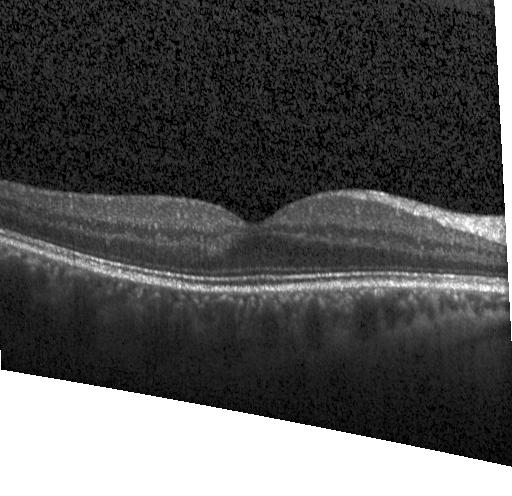
Finding: no evidence of choroidal neovascularization, diabetic macular edema, or drusen.